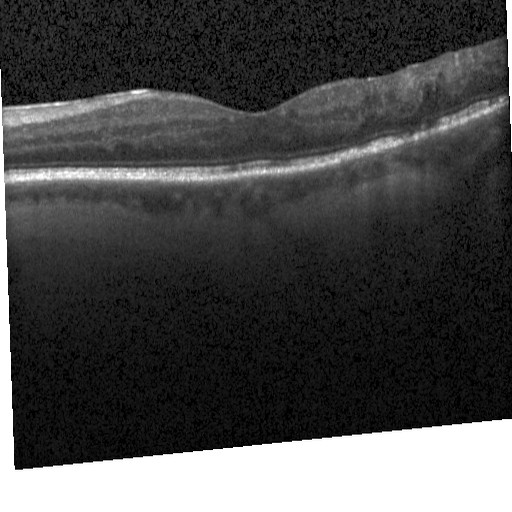
Spectral-domain optical coherence tomography; OCT B-scan; macular scan.
The scan shows diabetic macular edema.